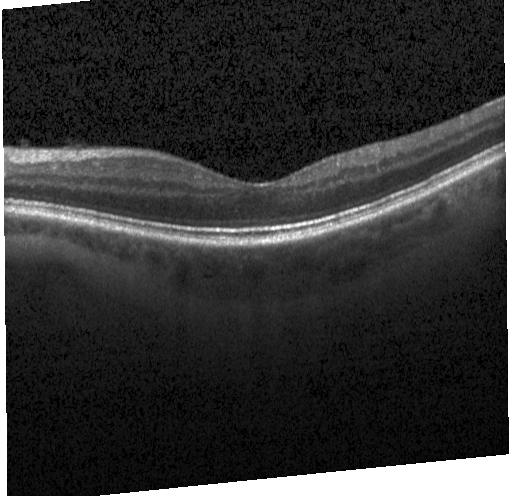

Through the macula. Acquired on a Heidelberg Spectralis. Optical coherence tomography B-scan — Macular OCT: no evidence of choroidal neovascularization, diabetic macular edema, or drusen.